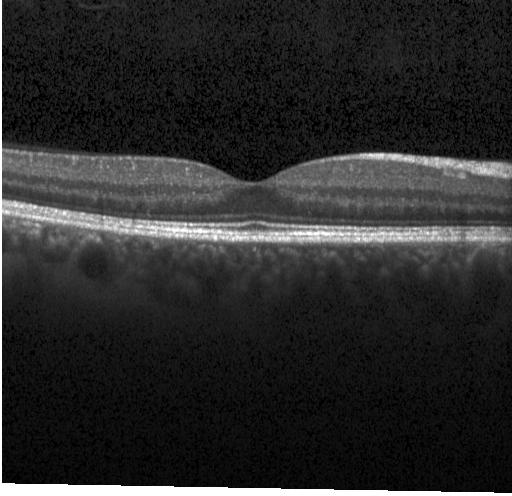
Acquired on a Heidelberg Spectralis; spectral-domain optical coherence tomography; optical coherence tomography B-scan.
Diagnosis: neither choroidal neovascularization, diabetic macular edema, nor drusen.